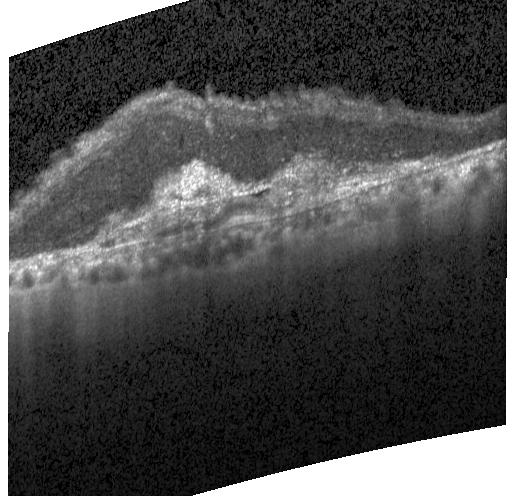

Retinal OCT cross-section.
The scan shows choroidal neovascularization (CNV).